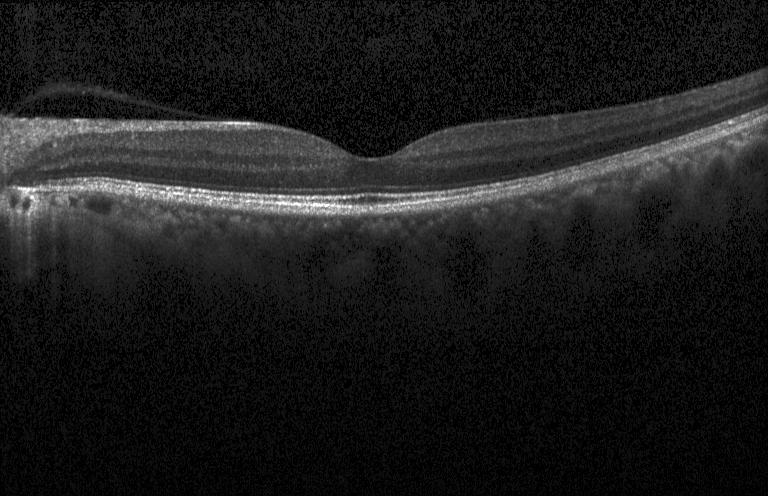
Retinal OCT cross-section showing neither choroidal neovascularization, diabetic macular edema, nor drusen.